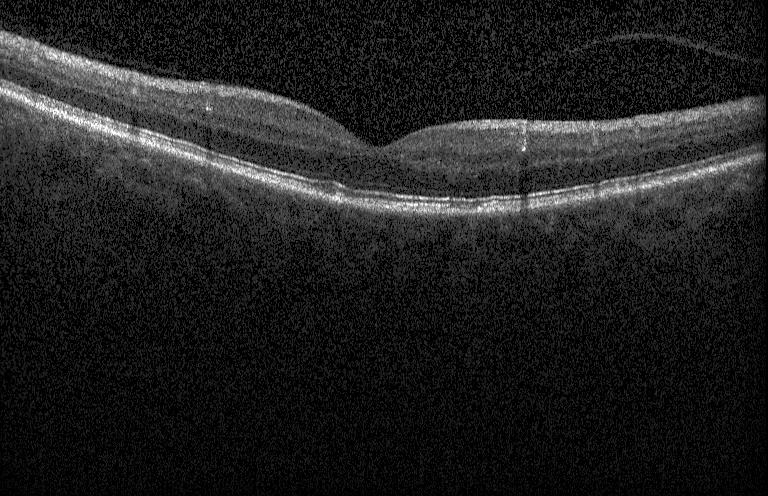

Dx: no choroidal neovascularization, no diabetic macular edema, and no drusen.